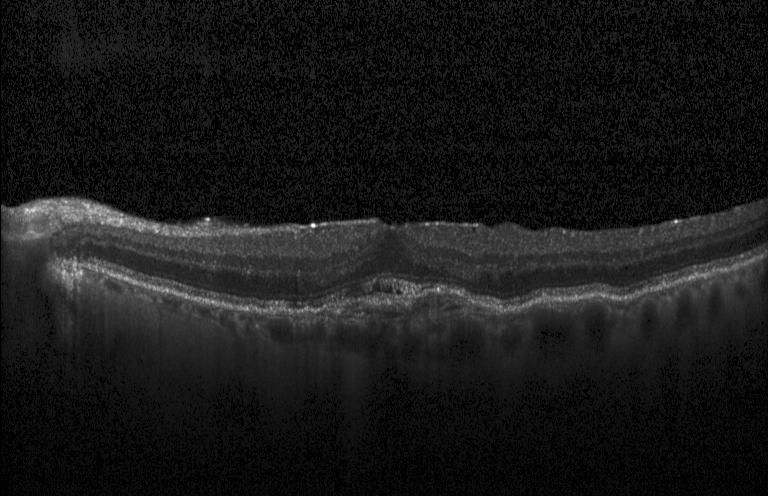 Diagnosis: CNV.